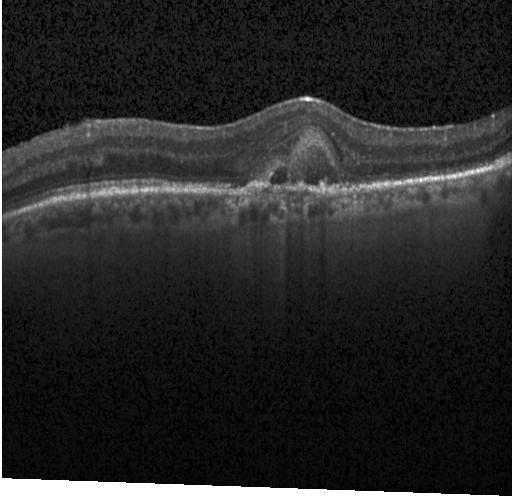
OCT B-scan, Heidelberg Spectralis.
The scan shows CNV.